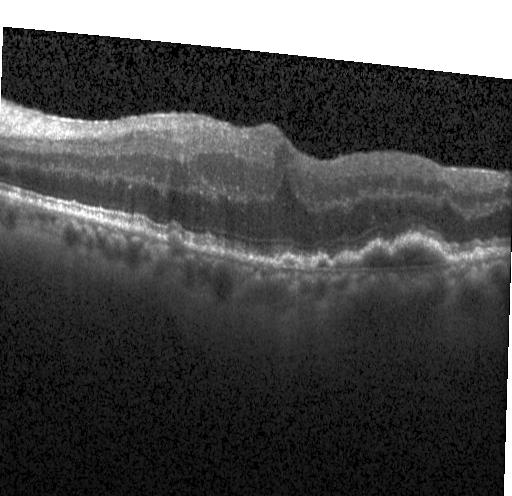 This B-scan demonstrates a choroidal neovascular membrane.